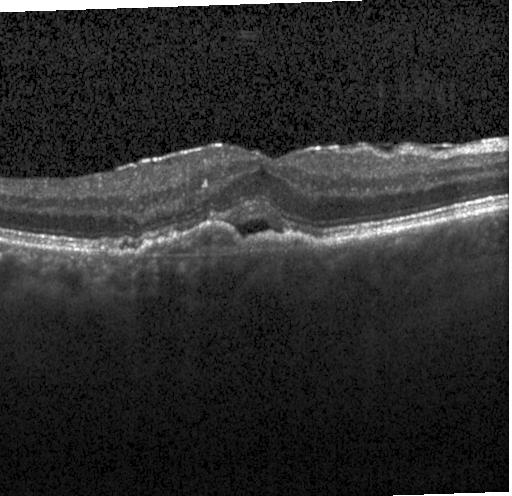
SD-OCT, centered on the fovea, OCT B-scan, instrument: Heidelberg Spectralis — Choroidal neovascularization (CNV).